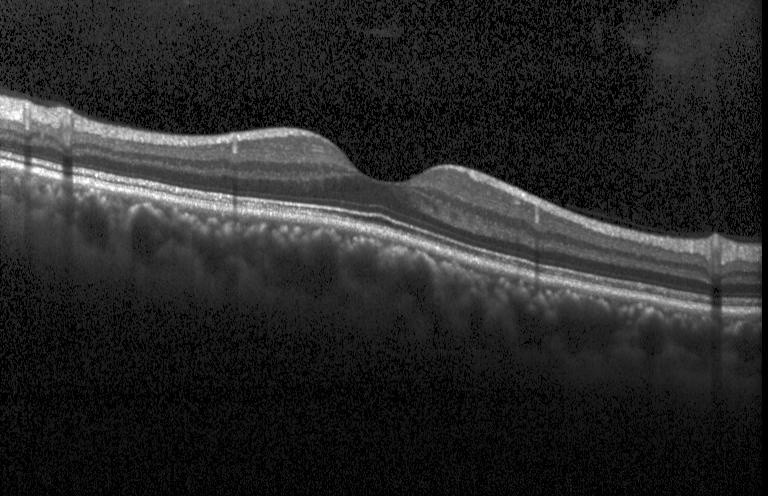

Fovea-centered, instrument: Heidelberg Spectralis, spectral-domain OCT, optical coherence tomography B-scan. OCT finding: no evidence of CNV, DME, or drusen.